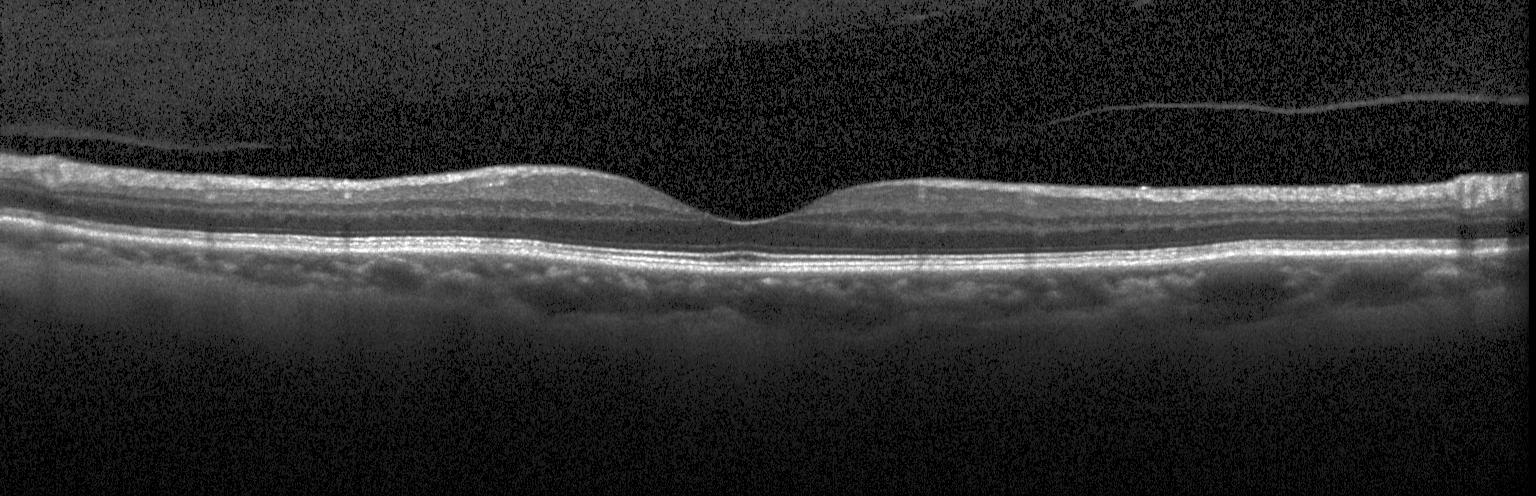

Impression: no choroidal neovascularization, diabetic macular edema, or drusen.